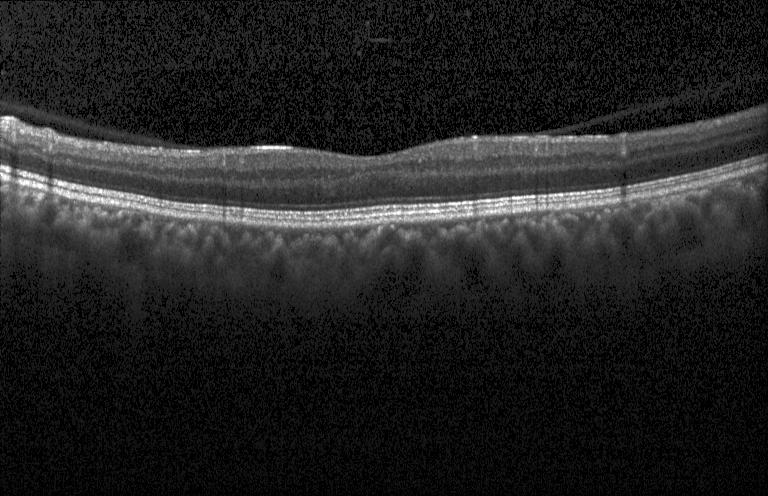 OCT B-scan showing no evidence of choroidal neovascularization, diabetic macular edema, or drusen.